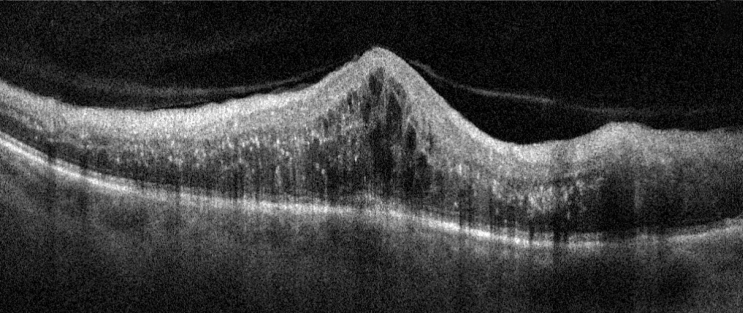
Optical coherence tomography scan
Impression: DME.